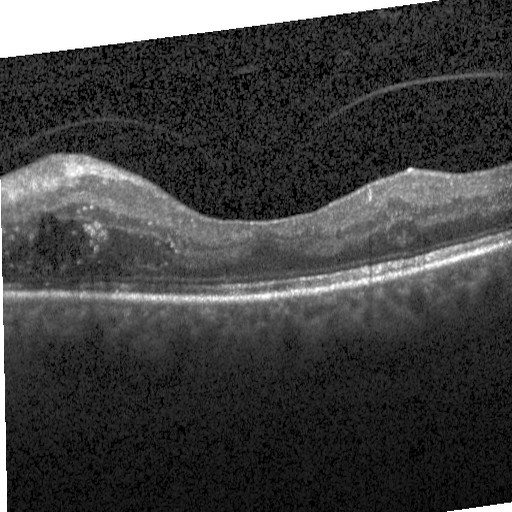 OCT B-scan showing DME.